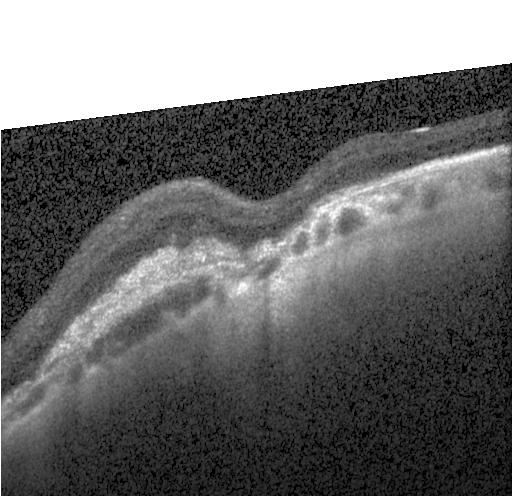 Retinal OCT cross-section showing a choroidal neovascular membrane.